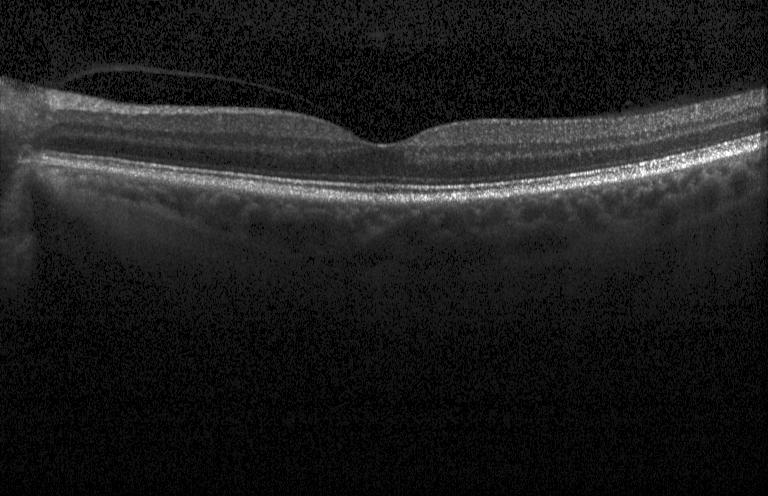

Acquired on a Heidelberg Spectralis · retinal OCT cross-section
Macular OCT: no CNV, DME, or drusen.